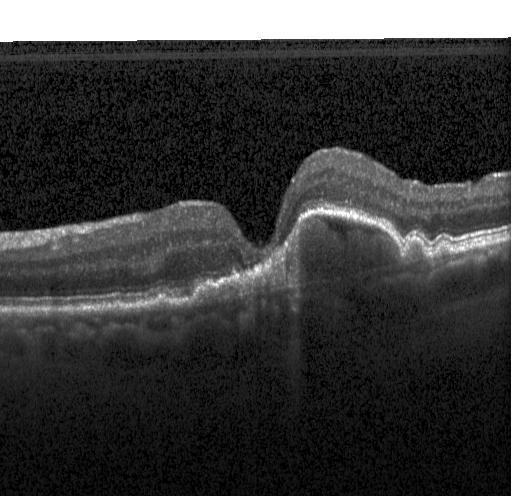 Horizontal scan through the fovea · optical coherence tomography scan · Heidelberg Spectralis. Dx: choroidal neovascularization (CNV).